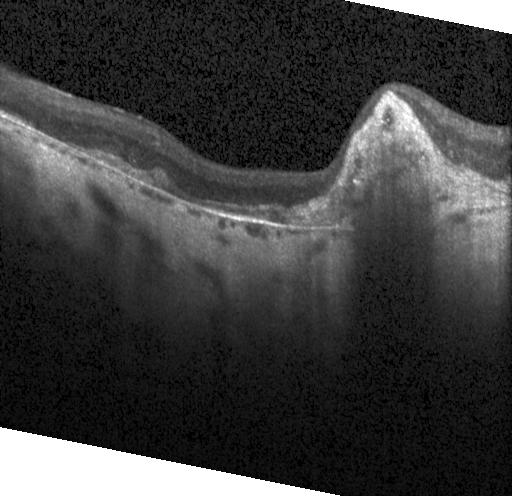
Fovea-centered; Heidelberg Spectralis OCT system; retinal OCT B-scan; spectral-domain optical coherence tomography.
This B-scan demonstrates a choroidal neovascular membrane.